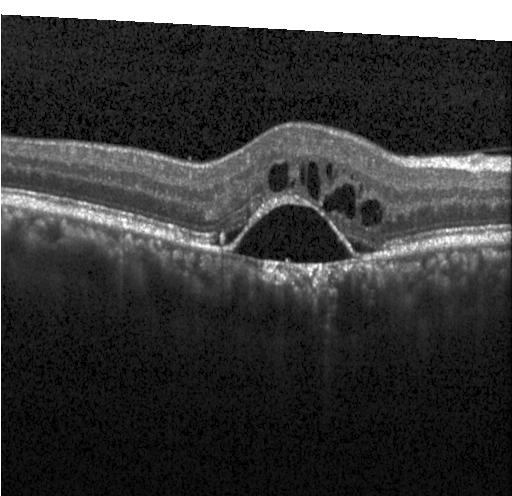
Impression: a choroidal neovascular membrane.